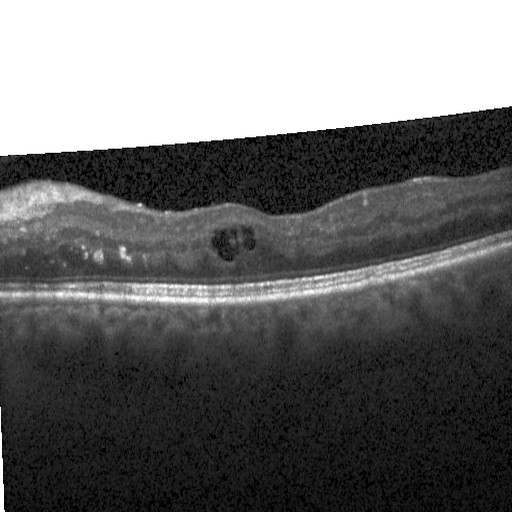 Finding: diabetic macular edema (DME).